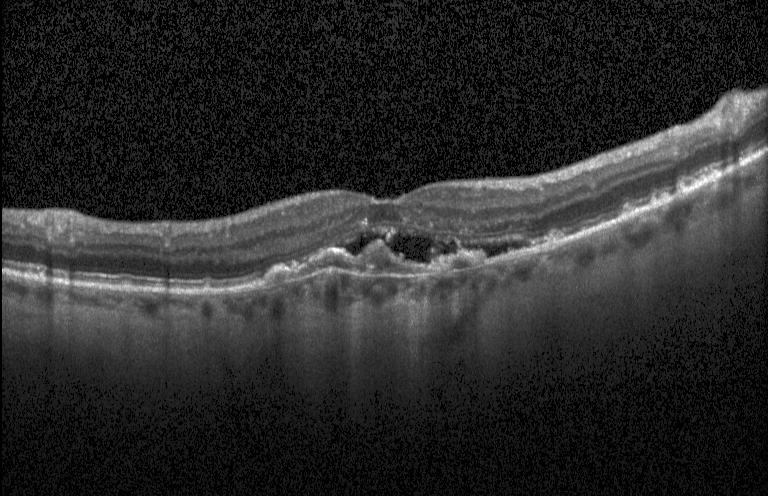 OCT scan showing a choroidal neovascular membrane.